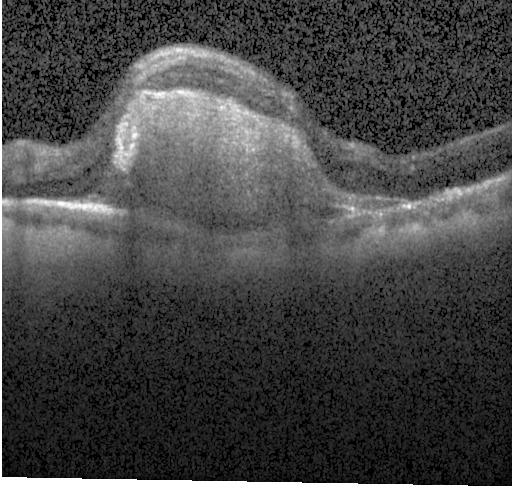
Optical coherence tomography scan; through the macula; Heidelberg Spectralis OCT system
Diagnosis: choroidal neovascularization.